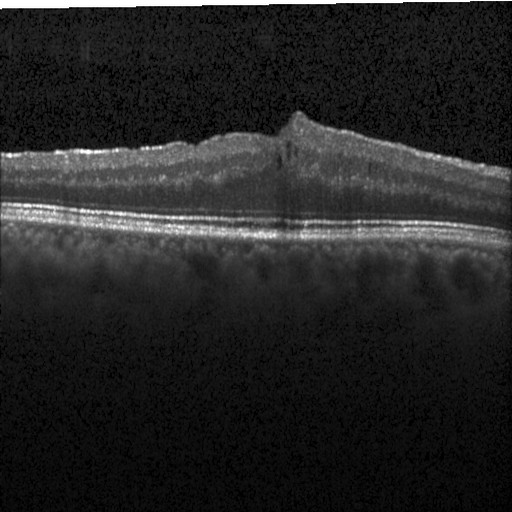 OCT B-scan showing DME.